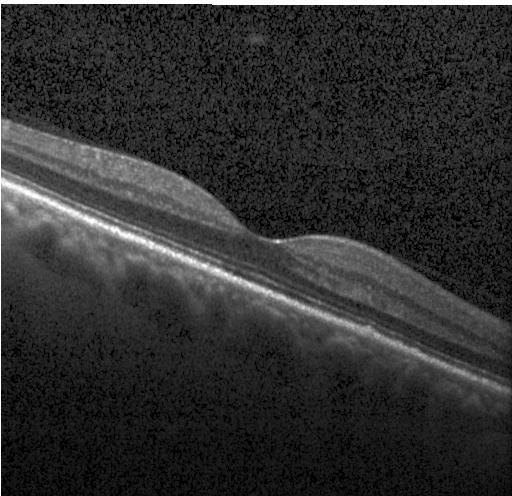 Heidelberg Spectralis OCT system · centered on the fovea · spectral-domain OCT · optical coherence tomography scan
Impression: no evidence of CNV, DME, or drusen.